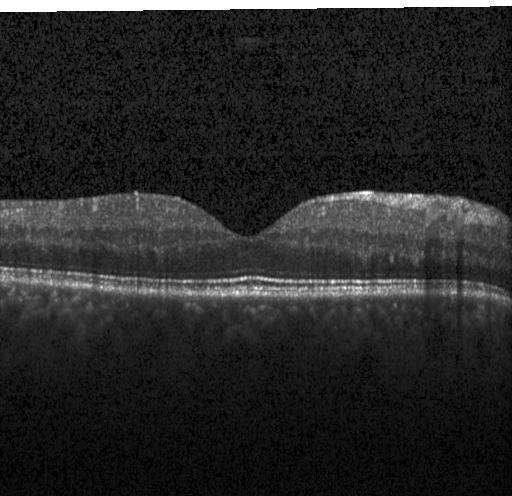
OCT line scan
The scan shows neither choroidal neovascularization, diabetic macular edema, nor drusen.